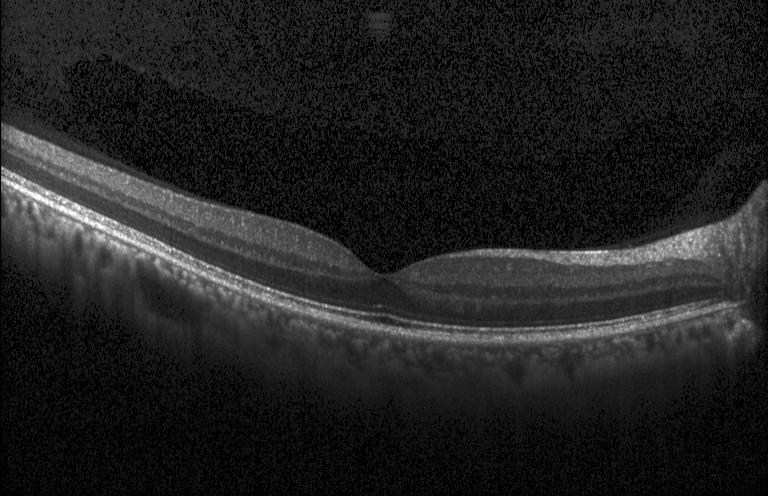
Impression: no choroidal neovascularization, no diabetic macular edema, and no drusen.